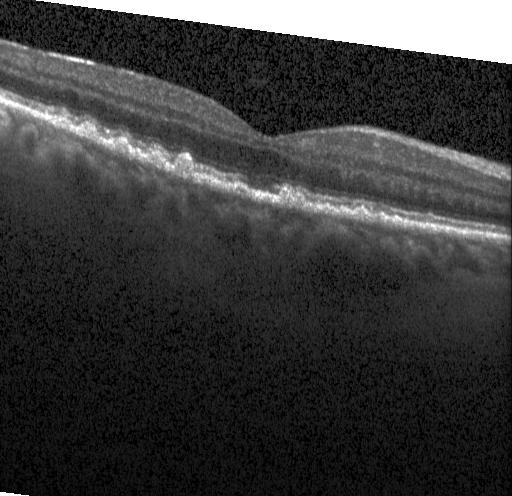 Macular OCT: sub-RPE drusenoid deposits.